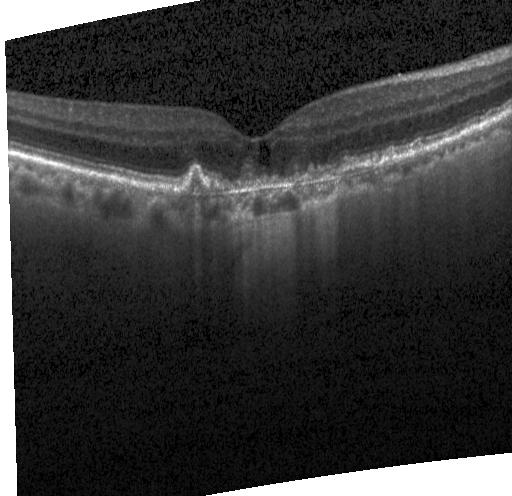
OCT B-scan showing a choroidal neovascular membrane.